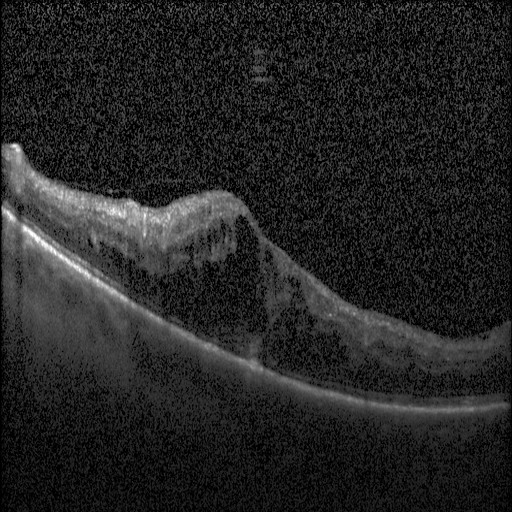

Acquired on a Heidelberg Spectralis; SD-OCT; optical coherence tomography B-scan; through the macula — Diagnosis: diabetic macular edema.